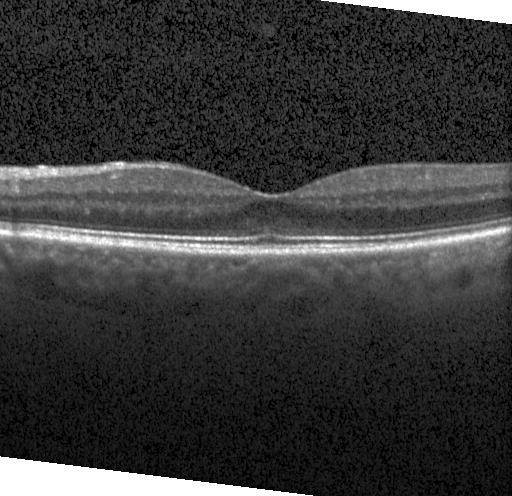 Spectral-domain optical coherence tomography. Retinal OCT cross-section — Diagnosis: neither choroidal neovascularization, diabetic macular edema, nor drusen.